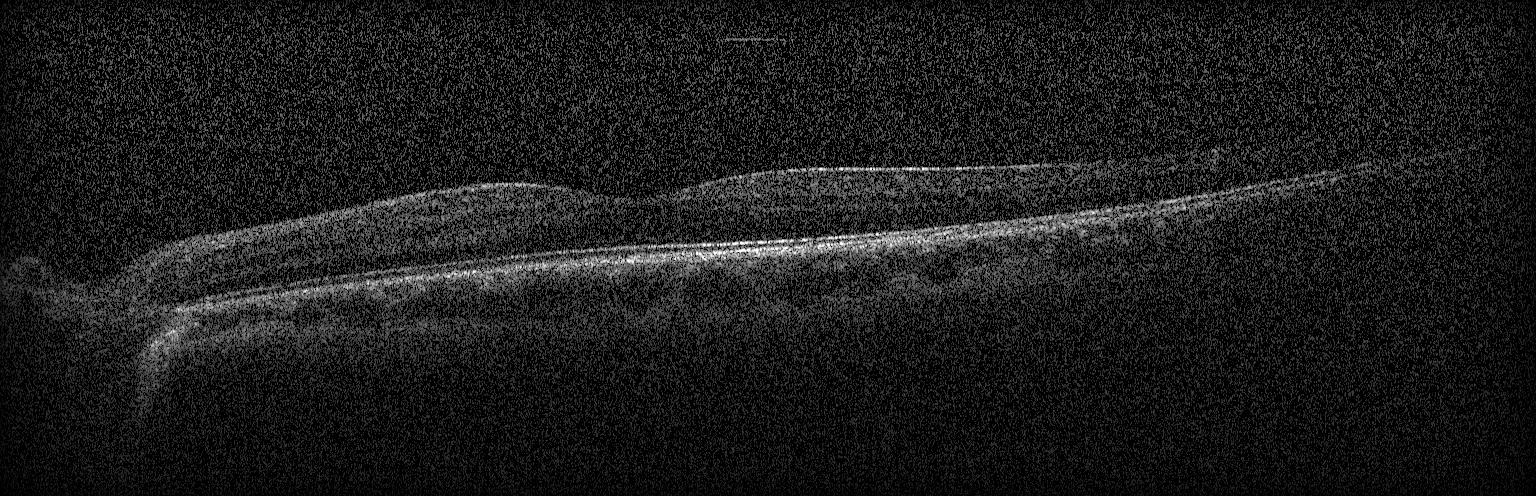 OCT scan showing neither CNV, DME, nor drusen.